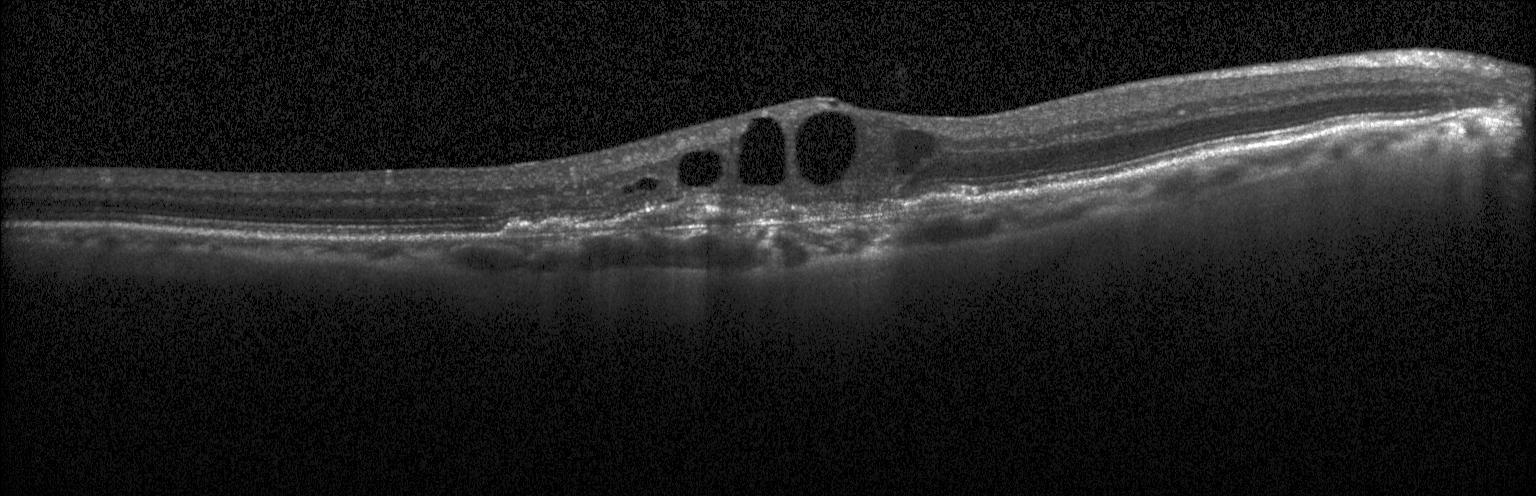

Optical coherence tomography scan. Instrument: Heidelberg Spectralis.
This B-scan demonstrates choroidal neovascularization.